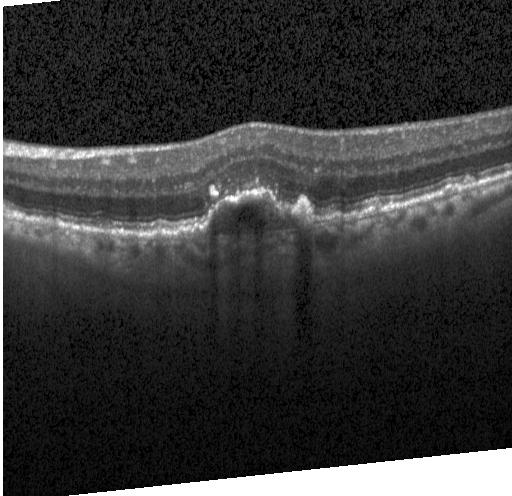

Optical coherence tomography scan. Assessment: a choroidal neovascular membrane.